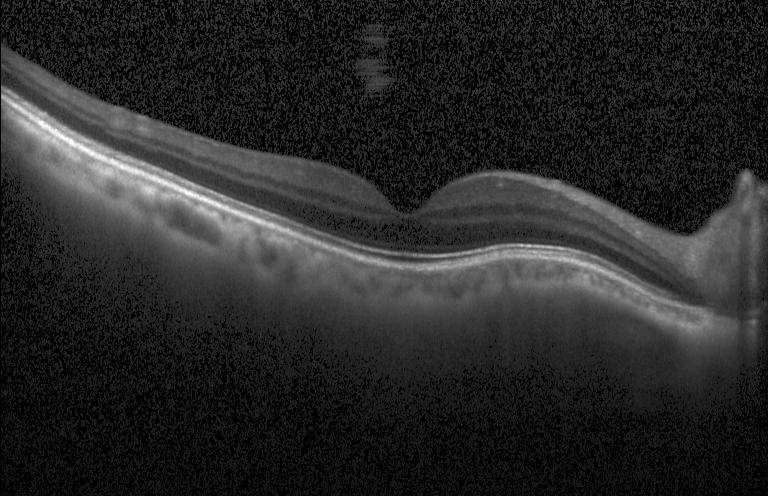

Optical coherence tomography scan, acquired on a Heidelberg Spectralis, spectral-domain optical coherence tomography, centered on the fovea — This B-scan demonstrates no choroidal neovascularization, no diabetic macular edema, and no drusen.